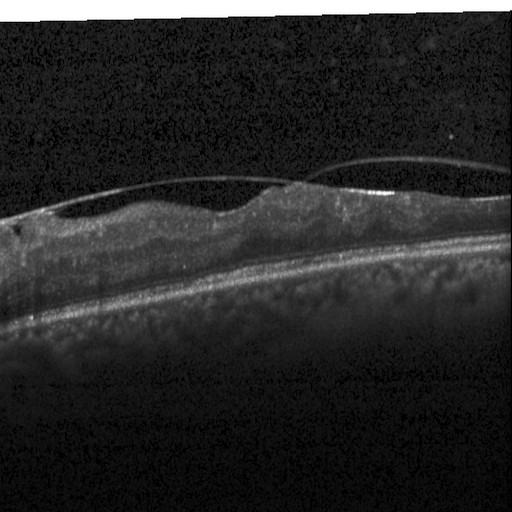

OCT finding: diabetic macular edema.